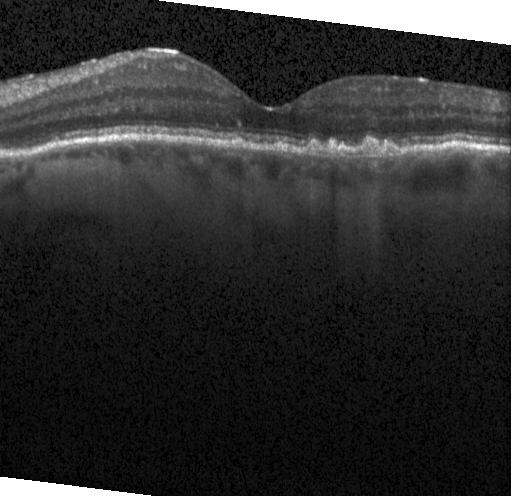
The scan shows sub-RPE drusenoid deposits.